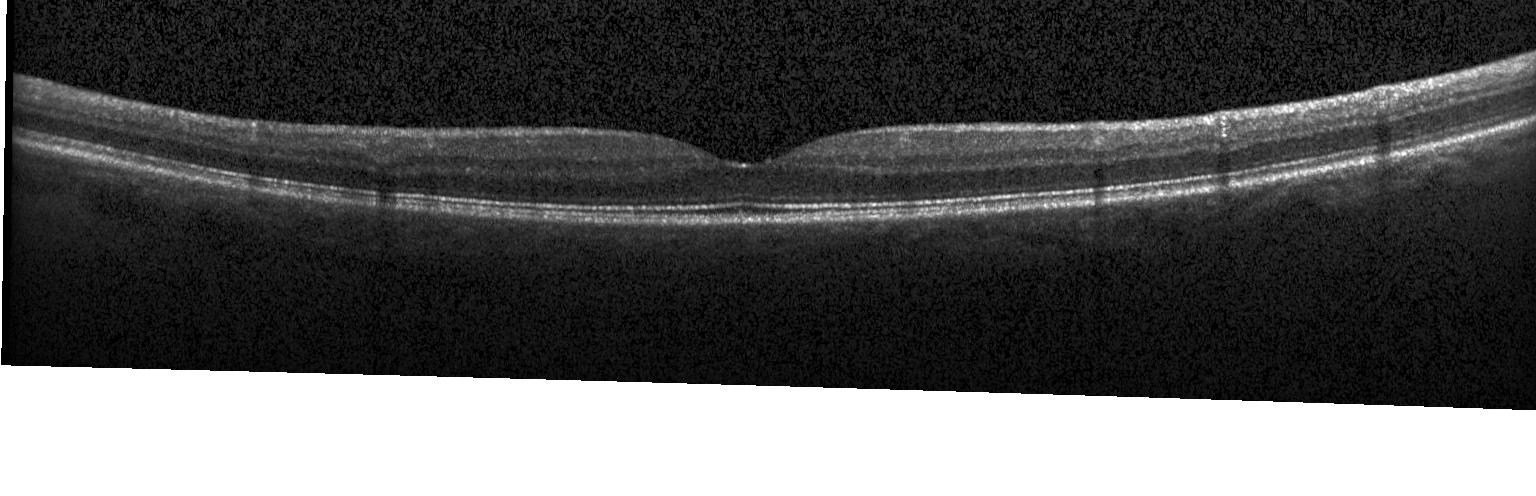 Dx: no choroidal neovascularization, no diabetic macular edema, and no drusen.